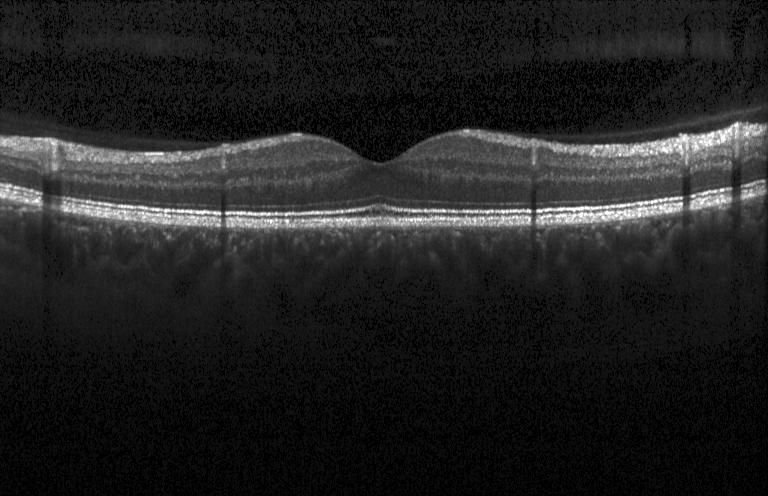 Spectral-domain optical coherence tomography; horizontal scan through the fovea; OCT line scan.
Dx: no CNV, DME, or drusen.